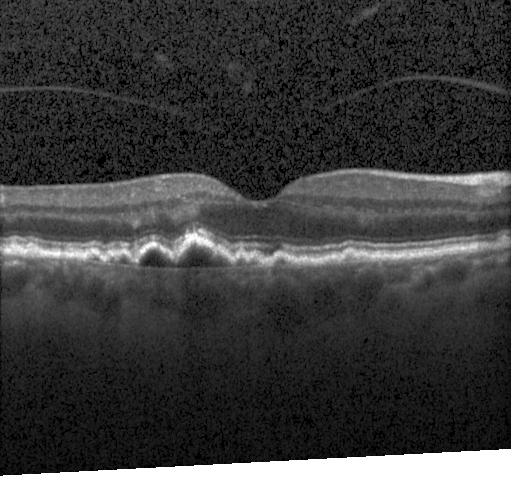

Acquired on a Heidelberg Spectralis. OCT B-scan. Spectral-domain OCT.
The scan shows a choroidal neovascular membrane.